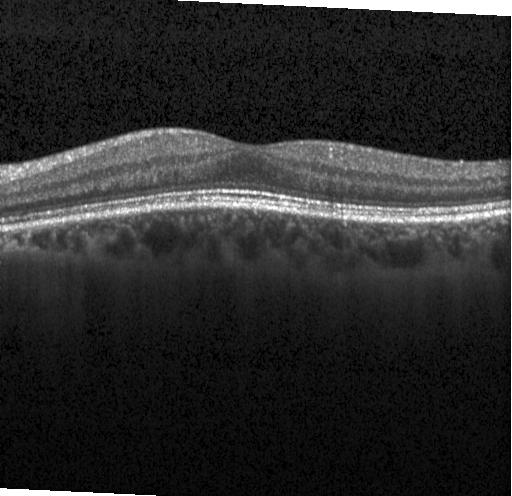 No CNV, no DME, and no drusen.